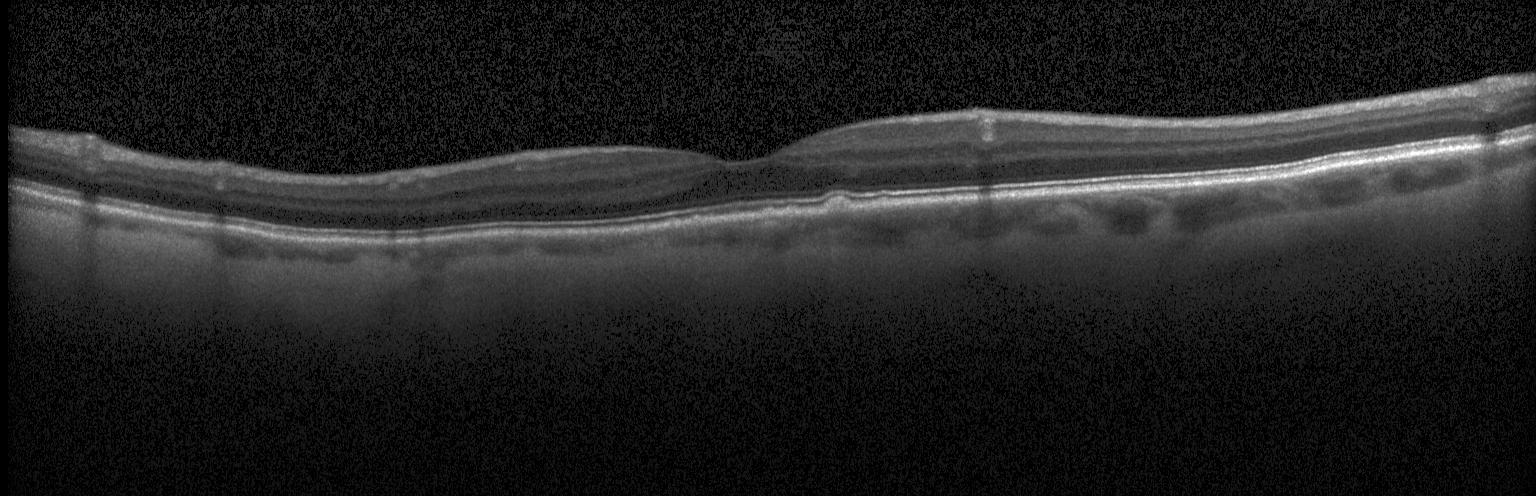

Macular OCT: multiple drusen.